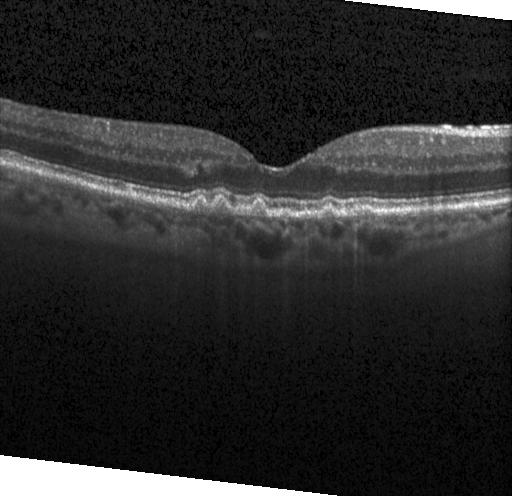 Optical coherence tomography scan.
Impression: multiple drusen.